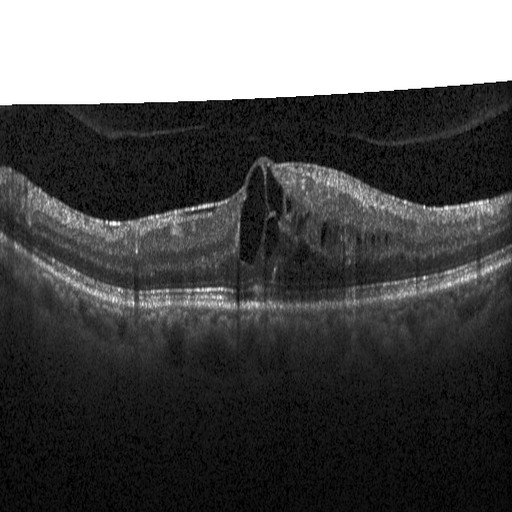 Instrument: Heidelberg Spectralis · through the macula · retinal OCT B-scan · spectral-domain OCT.
OCT finding: diabetic macular edema.